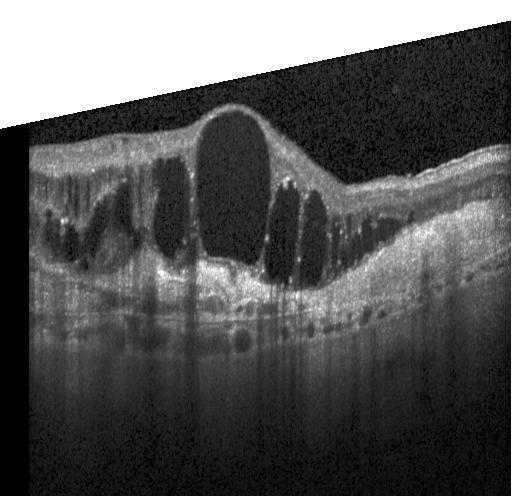
Spectral-domain OCT B-scan: a choroidal neovascular membrane.